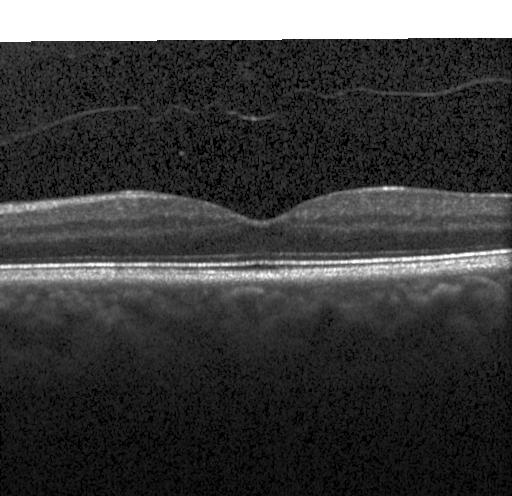
OCT B-scan; Heidelberg Spectralis OCT system; spectral-domain optical coherence tomography; through the macula — Finding: no choroidal neovascularization, no diabetic macular edema, and no drusen.